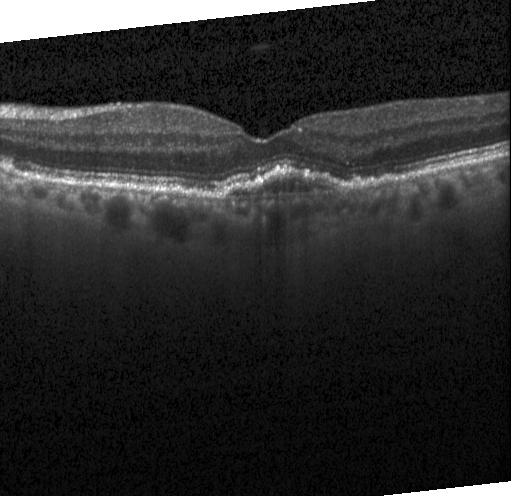

Optical coherence tomography B-scan.
A choroidal neovascular membrane.